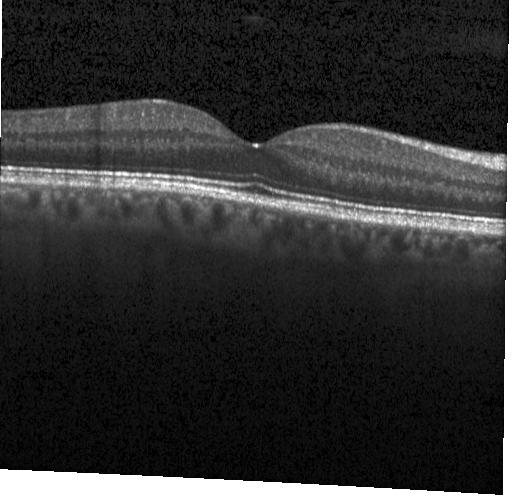
Finding: no CNV, no DME, and no drusen.